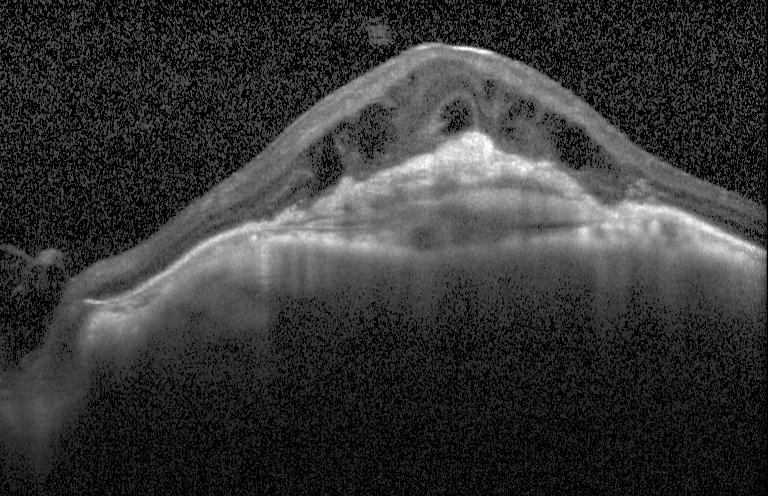 Fovea-centered · optical coherence tomography scan · spectral-domain optical coherence tomography
Impression: a choroidal neovascular membrane.